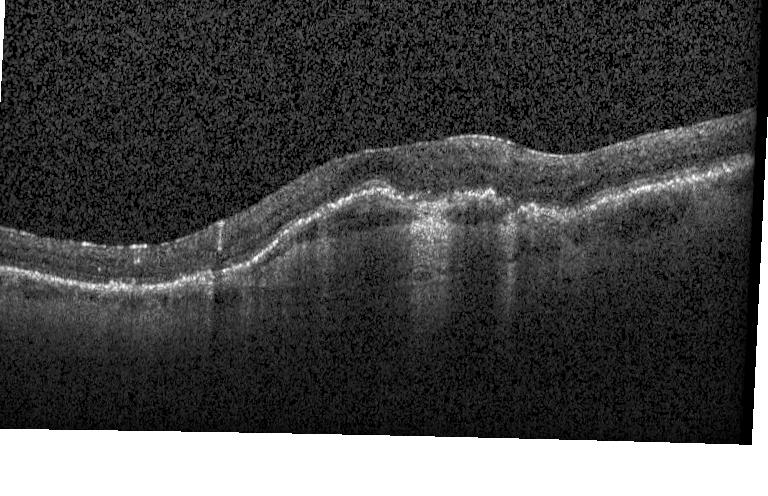 OCT B-scan; acquired on a Heidelberg Spectralis; macular scan. Assessment: choroidal neovascularization.